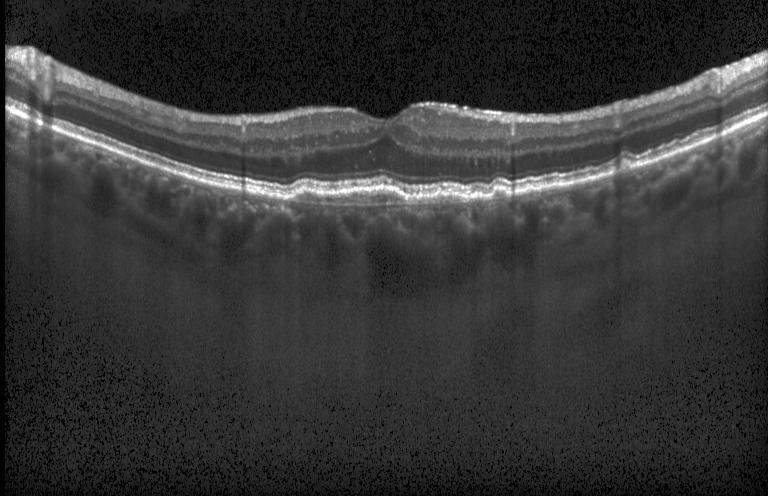 Retinal OCT B-scan · Heidelberg Spectralis OCT system.
Finding: CNV.